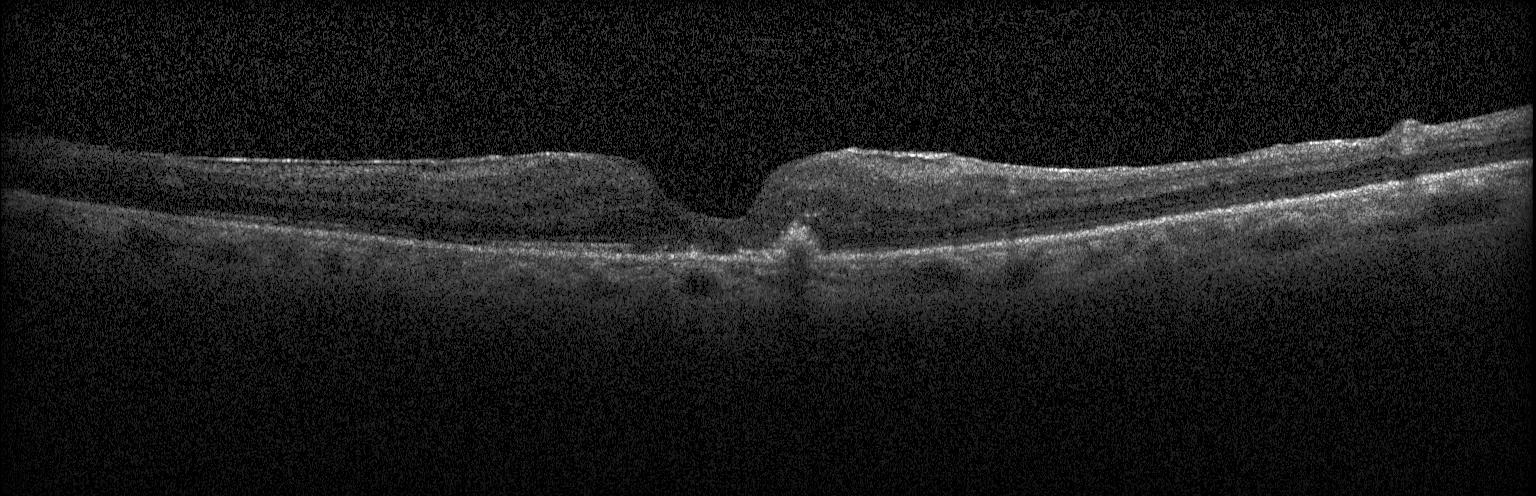

Spectral-domain OCT B-scan: drusen.